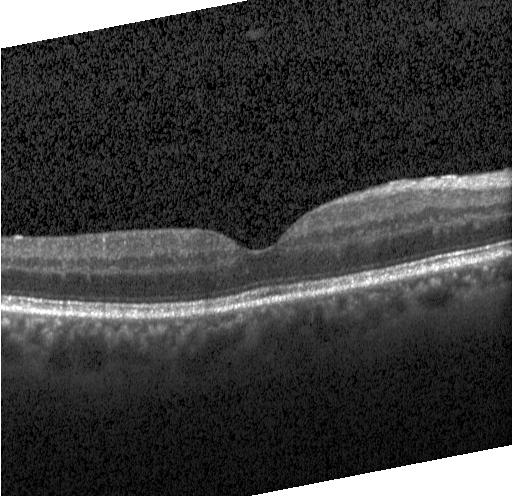
Diagnosis: neither choroidal neovascularization, diabetic macular edema, nor drusen.